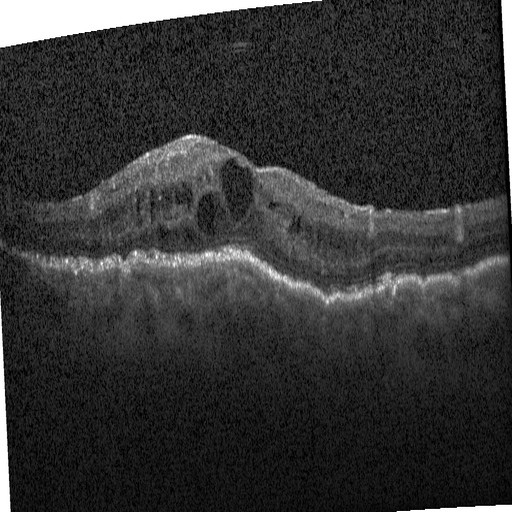 OCT B-scan — OCT finding: DME.